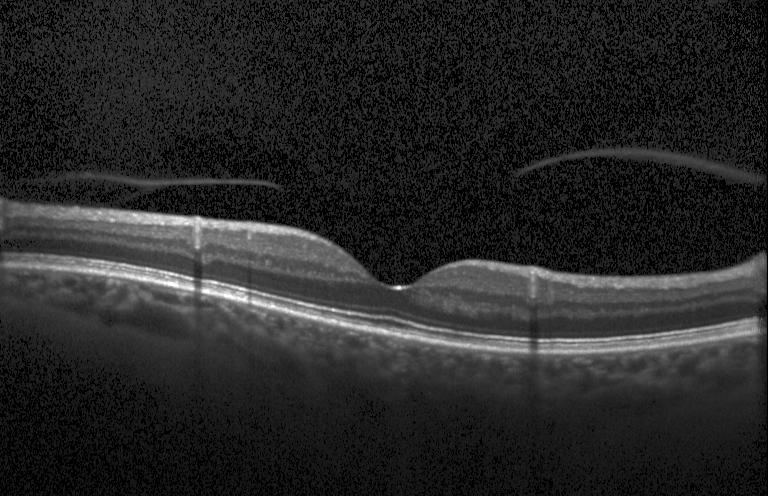 The scan shows neither CNV, DME, nor drusen.